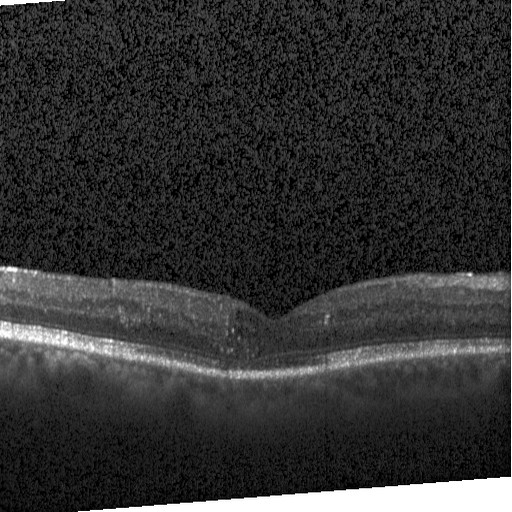
Macular OCT demonstrating diabetic macular edema (DME).